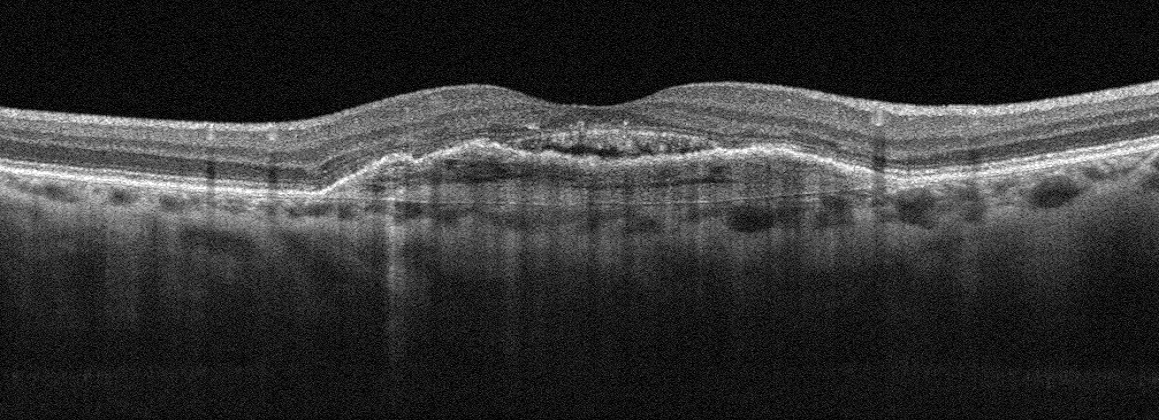 Retinal OCT B-scan; Optovue Avanti RTVue XR; oculus dexter
This B-scan demonstrates AMD.